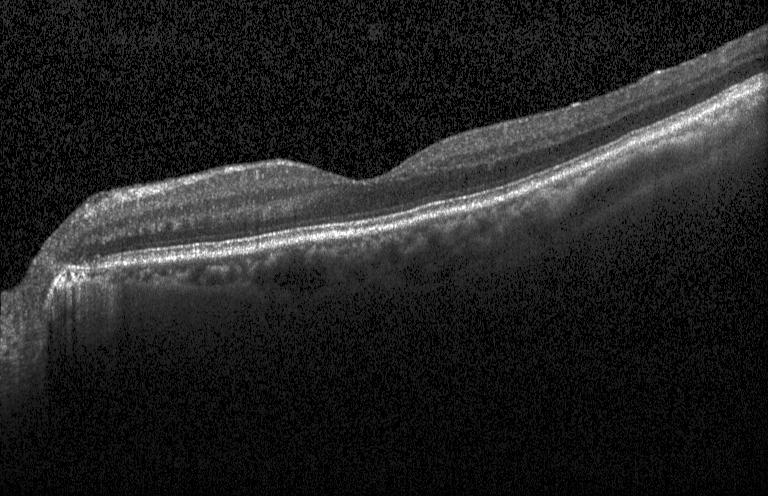
Diagnosis: no CNV, DME, or drusen.